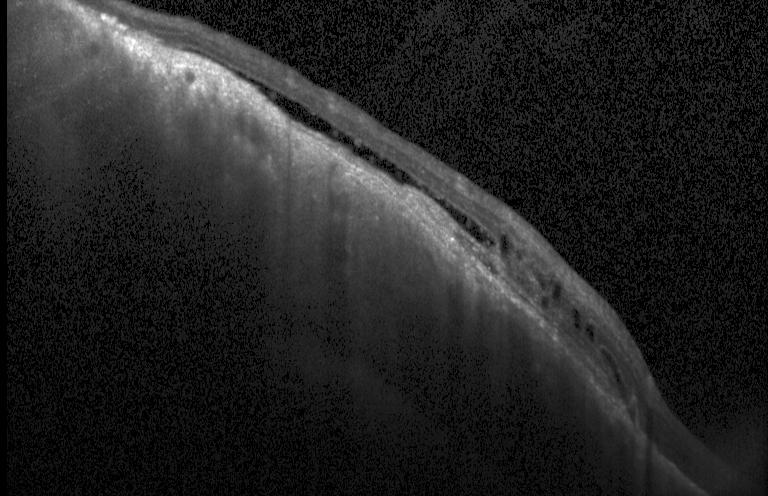

OCT scan showing a choroidal neovascular membrane.